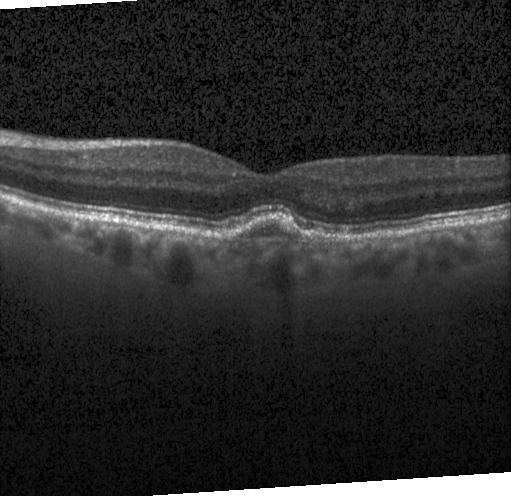
Heidelberg Spectralis OCT system. Spectral-domain OCT. OCT line scan. Fovea-centered — Finding: choroidal neovascularization (CNV).